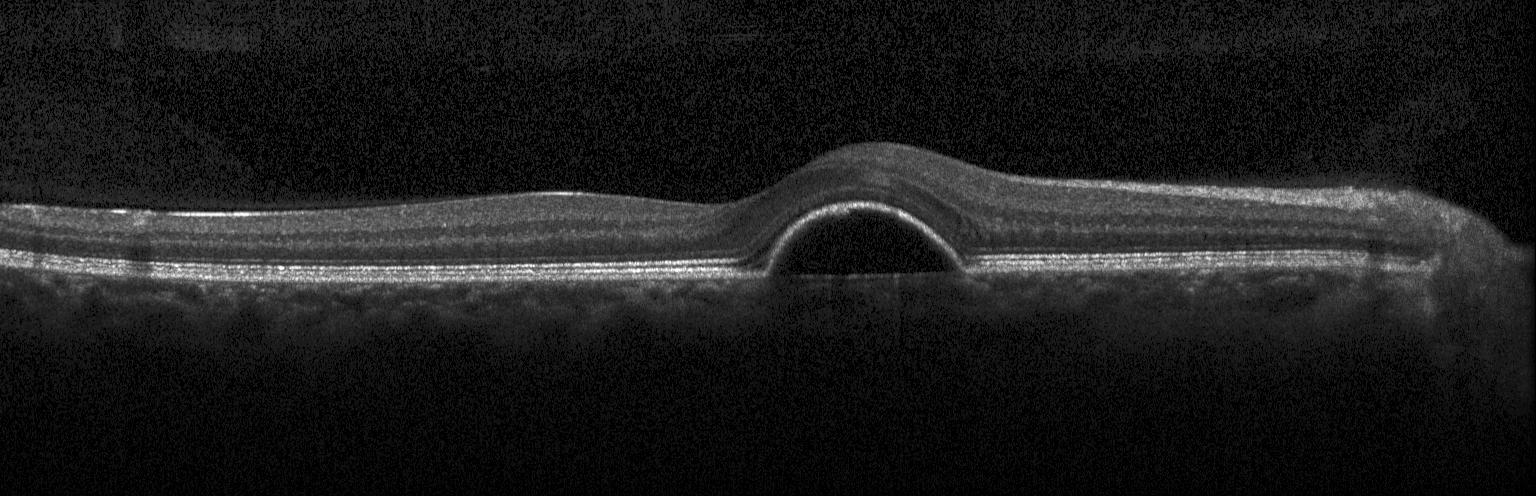
Retinal OCT B-scan; centered on the fovea; SD-OCT; acquired on a Heidelberg Spectralis — Impression: a choroidal neovascular membrane.